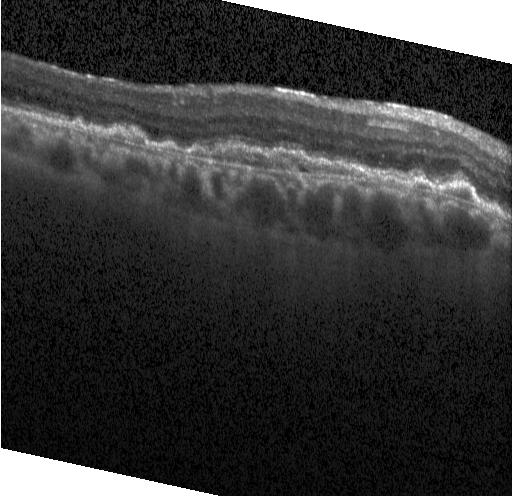

Assessment: choroidal neovascularization.